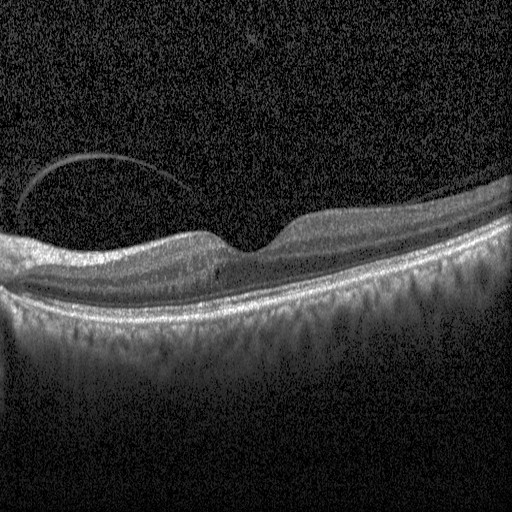 Spectral-domain OCT. Centered on the fovea. Acquired on a Heidelberg Spectralis. Optical coherence tomography B-scan — Diagnosis: DME.